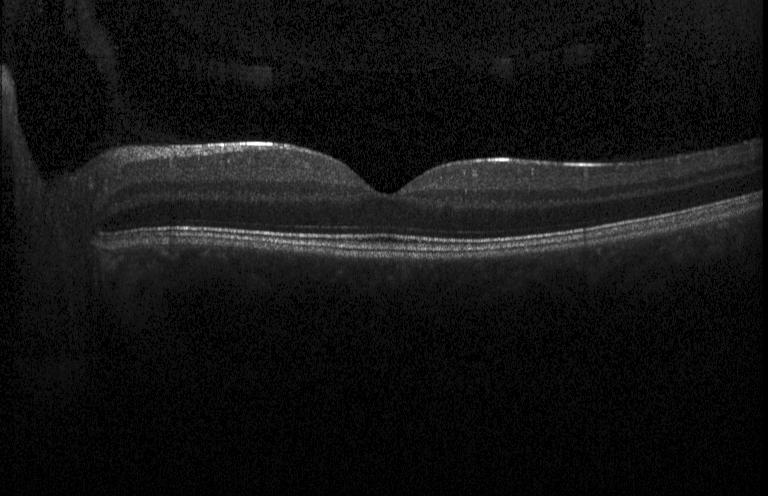 OCT line scan, Heidelberg Spectralis OCT system.
No CNV, no DME, and no drusen.